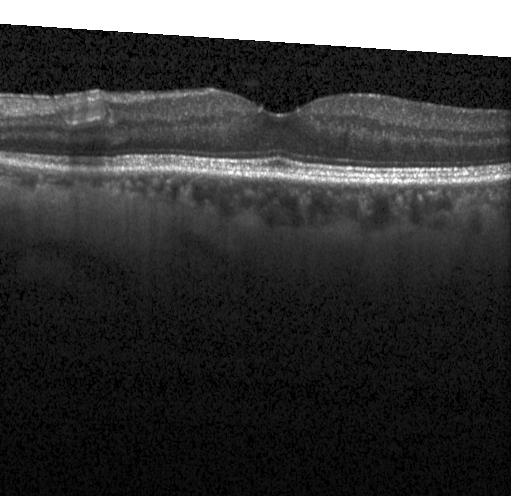

Retinal OCT cross-section, spectral-domain OCT, through the macula. Finding: no choroidal neovascularization, diabetic macular edema, or drusen.